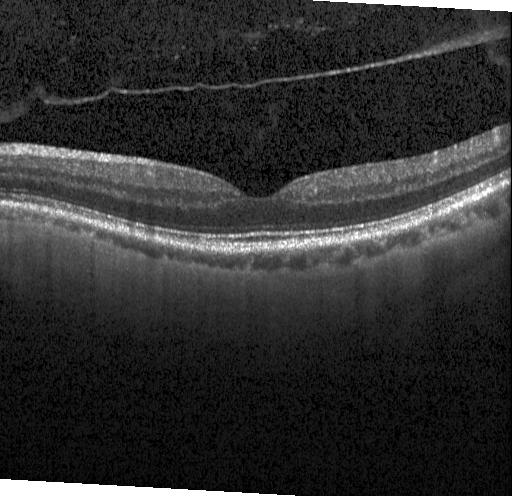

OCT line scan, spectral-domain OCT, instrument: Heidelberg Spectralis
Diagnosis: no choroidal neovascularization, no diabetic macular edema, and no drusen.